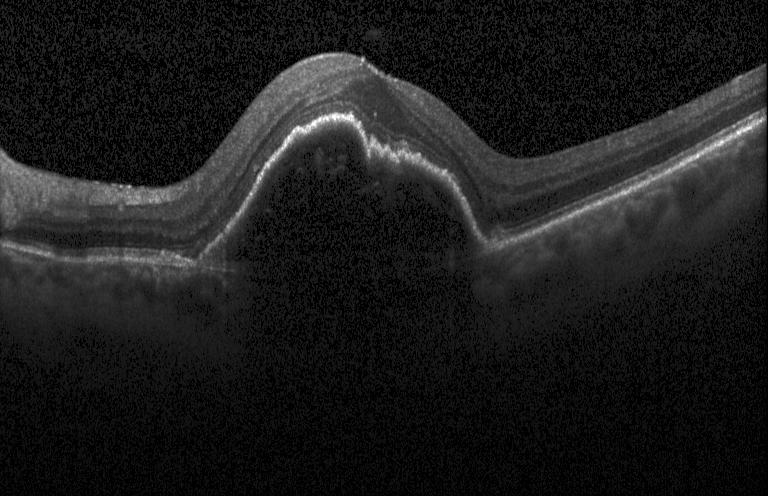

Retinal OCT B-scan — Dx: choroidal neovascularization (CNV).